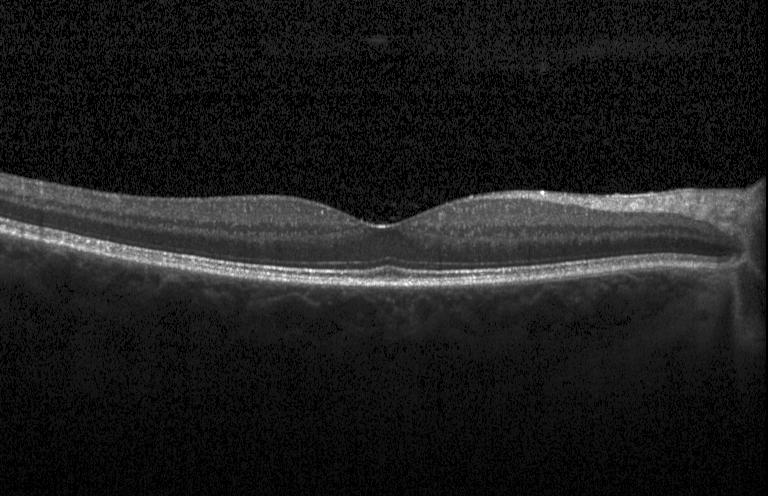
Retinal OCT cross-section showing no CNV, DME, or drusen.